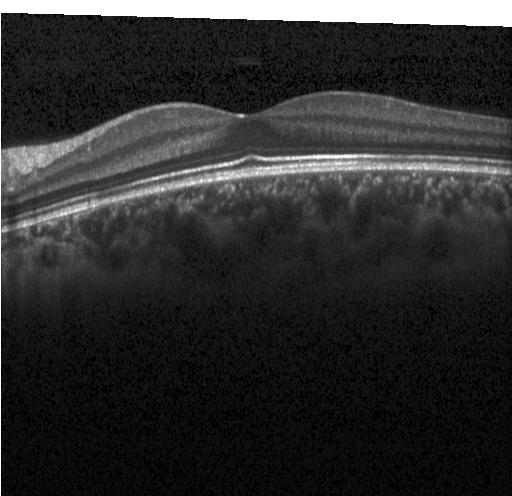

Finding: no evidence of choroidal neovascularization, diabetic macular edema, or drusen.